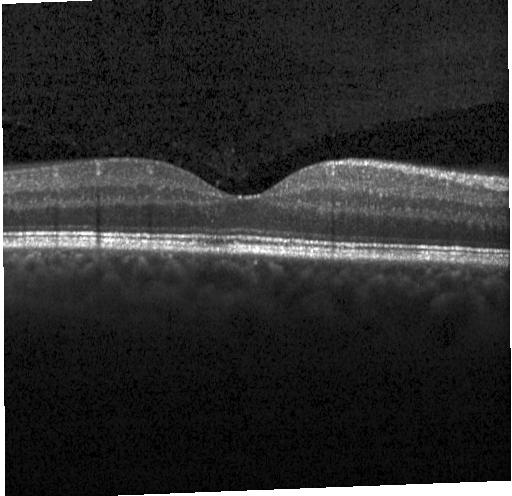 Fovea-centered, OCT B-scan.
OCT finding: no evidence of choroidal neovascularization, diabetic macular edema, or drusen.